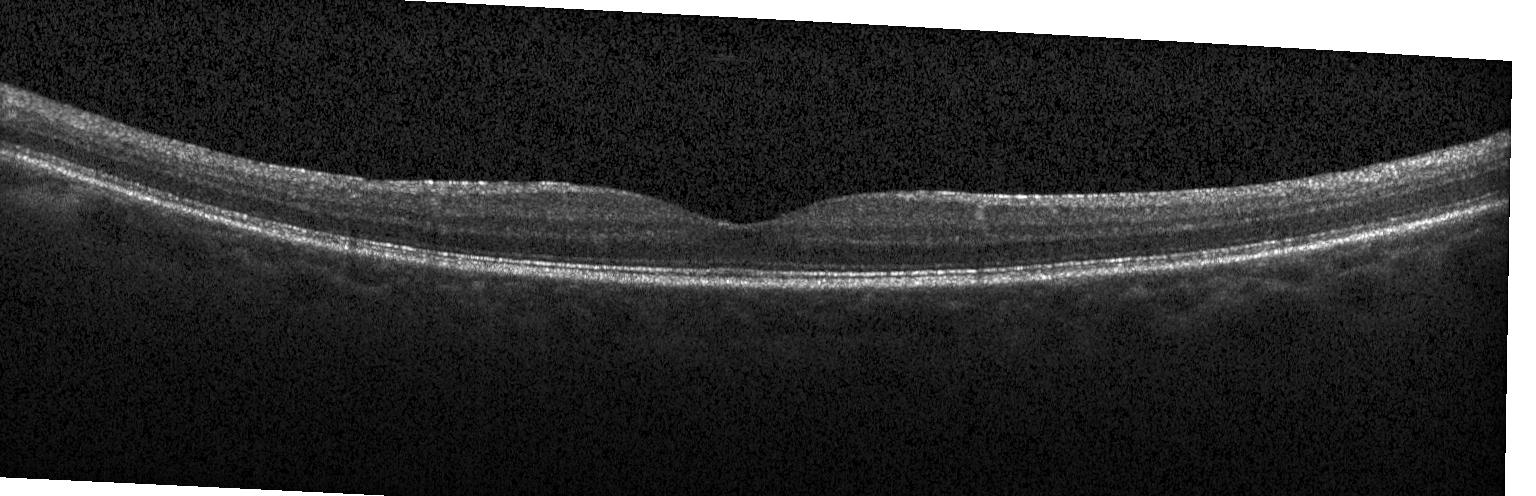
Instrument: Heidelberg Spectralis; horizontal scan through the fovea; optical coherence tomography B-scan. The scan shows no choroidal neovascularization, diabetic macular edema, or drusen.